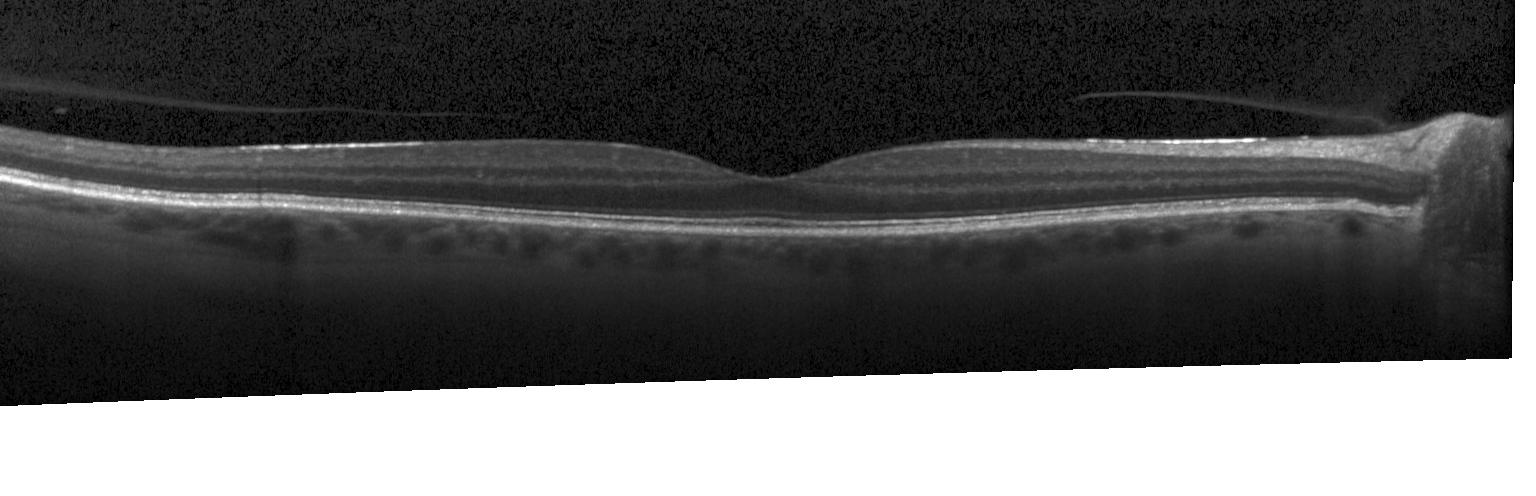
Macular OCT demonstrating neither choroidal neovascularization, diabetic macular edema, nor drusen.